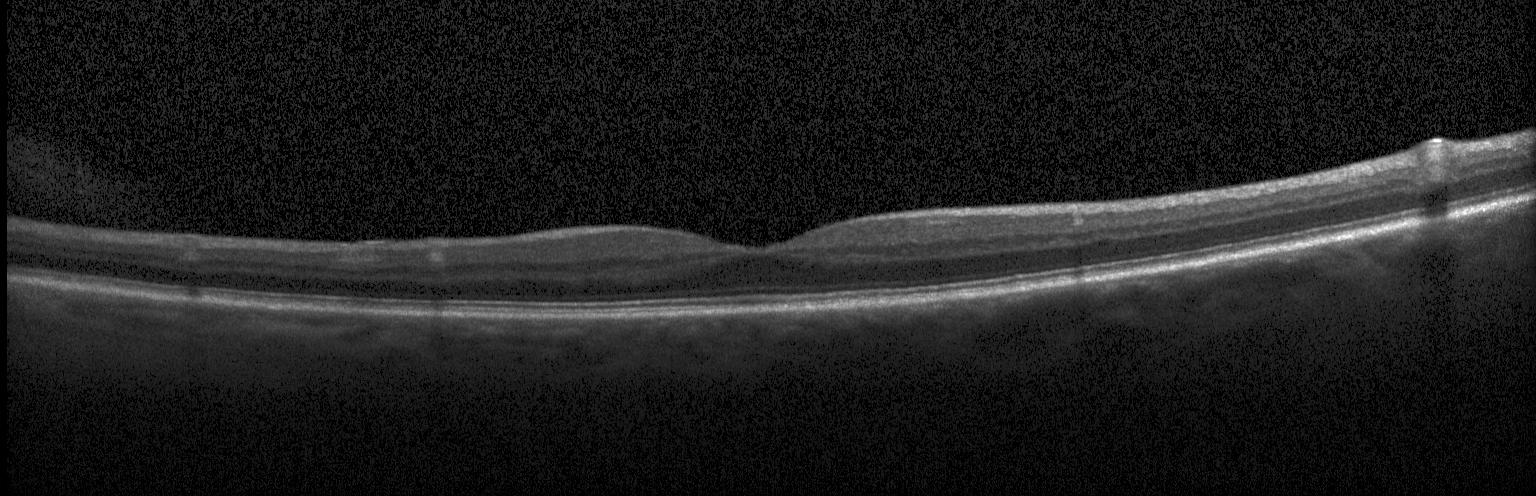 OCT line scan. Dx: no CNV, no DME, and no drusen.